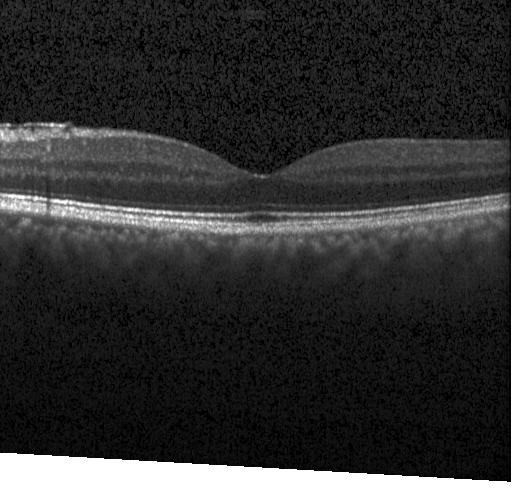

Retinal OCT B-scan
Dx: no evidence of CNV, DME, or drusen.